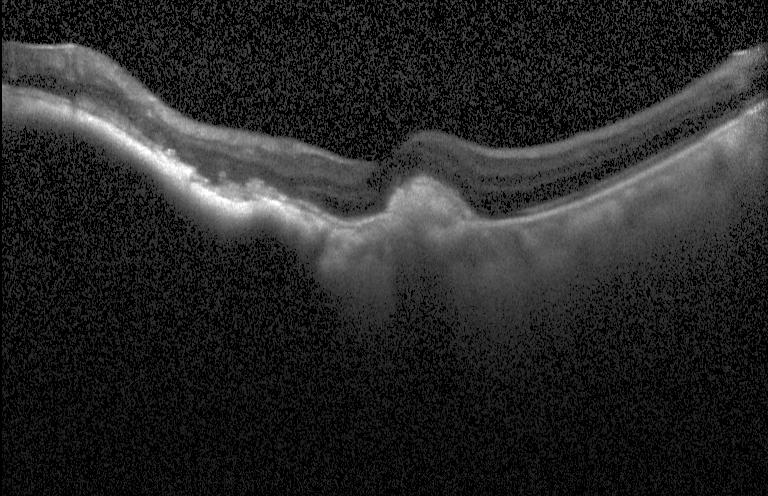

Heidelberg Spectralis. Retinal OCT B-scan — Impression: choroidal neovascularization (CNV).